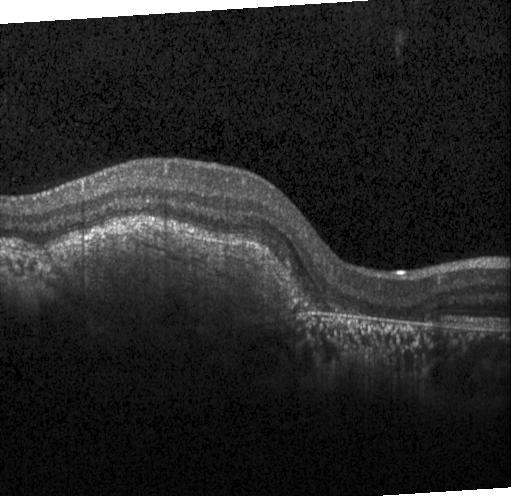
OCT line scan. Through the macula.
Macular OCT: choroidal neovascularization (CNV).